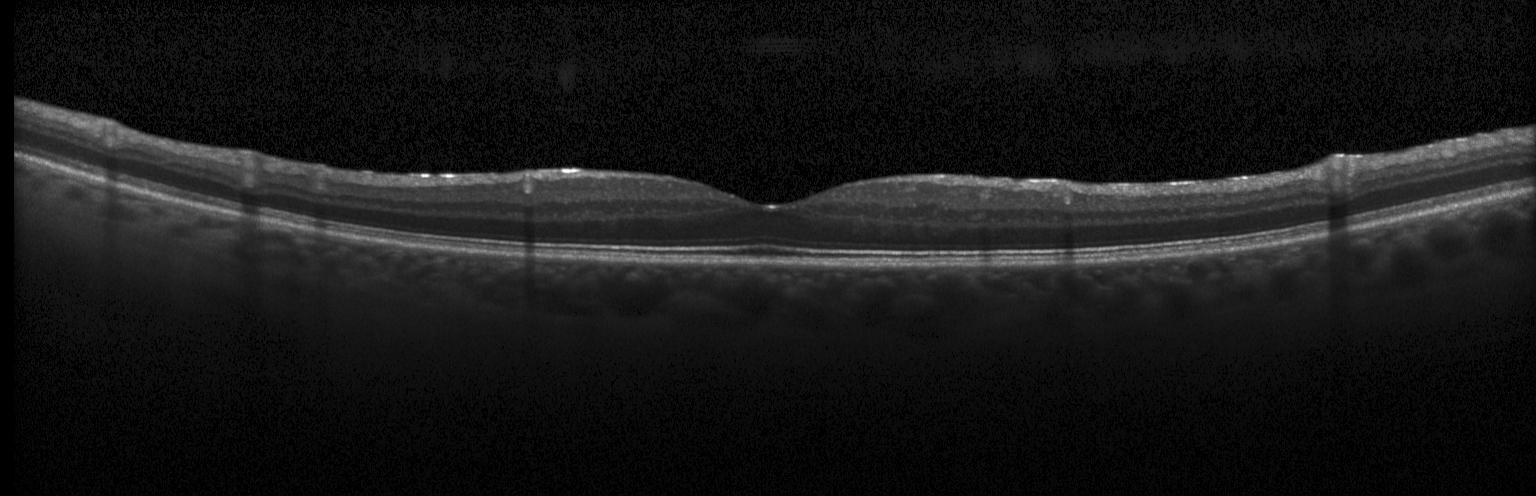 Impression: no CNV, no DME, and no drusen.